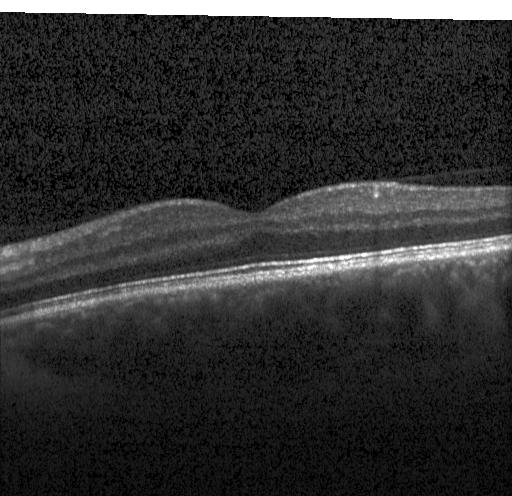

OCT line scan; spectral-domain optical coherence tomography; instrument: Heidelberg Spectralis; macular scan — Impression: no choroidal neovascularization, no diabetic macular edema, and no drusen.